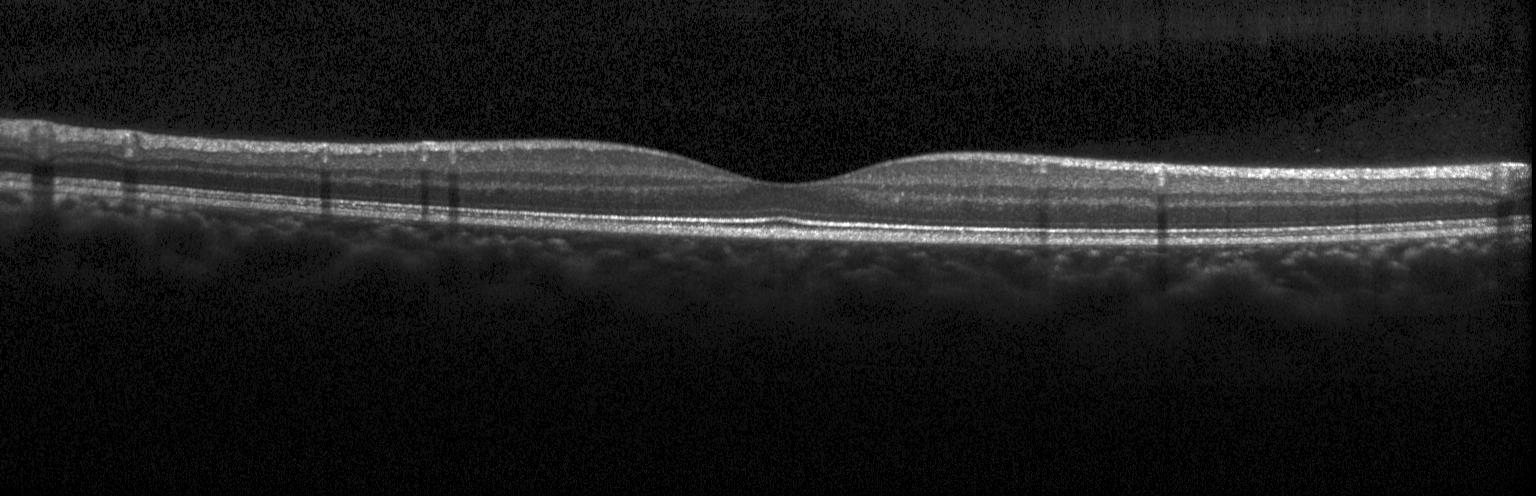 Macular OCT: no choroidal neovascularization, no diabetic macular edema, and no drusen.